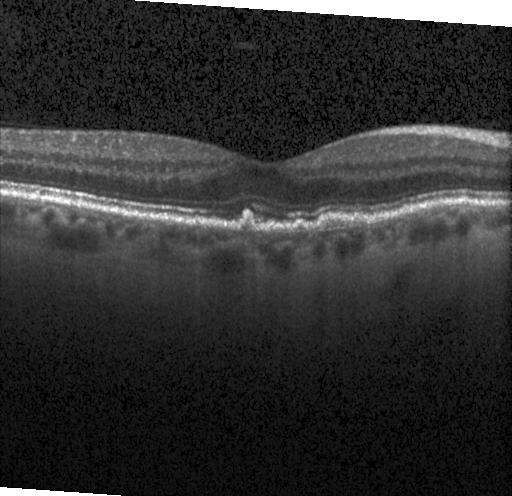

Finding: drusen.